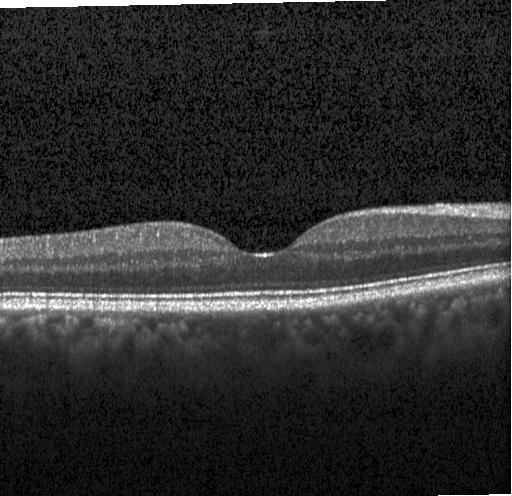

OCT line scan, acquired on a Heidelberg Spectralis.
Diagnosis: no evidence of choroidal neovascularization, diabetic macular edema, or drusen.